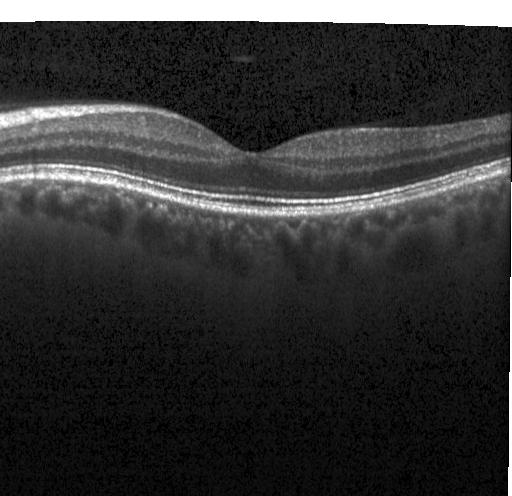 Finding: no evidence of choroidal neovascularization, diabetic macular edema, or drusen.